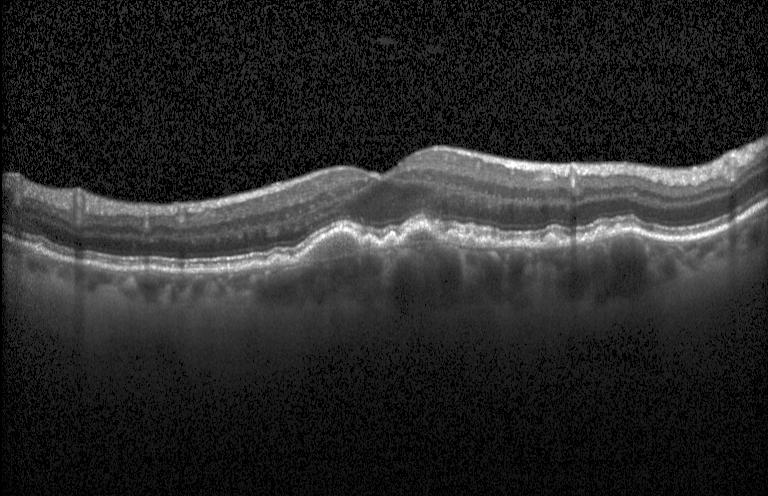 Diagnosis: sub-RPE drusenoid deposits.